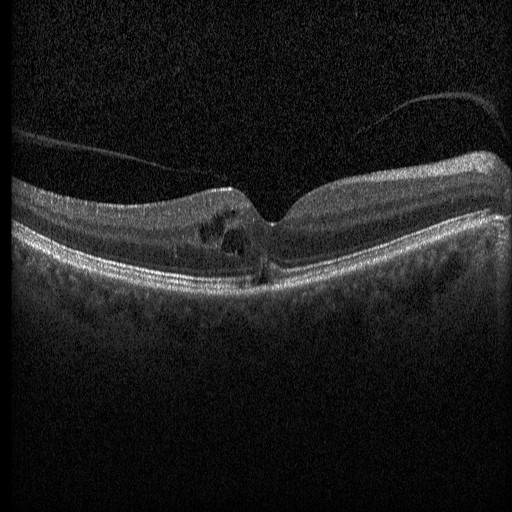
Heidelberg Spectralis OCT system. Retinal OCT cross-section — OCT finding: DME.